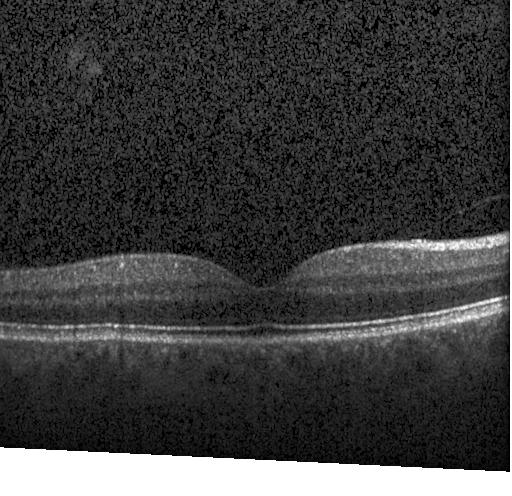
Retinal OCT B-scan.
No CNV, no DME, and no drusen.